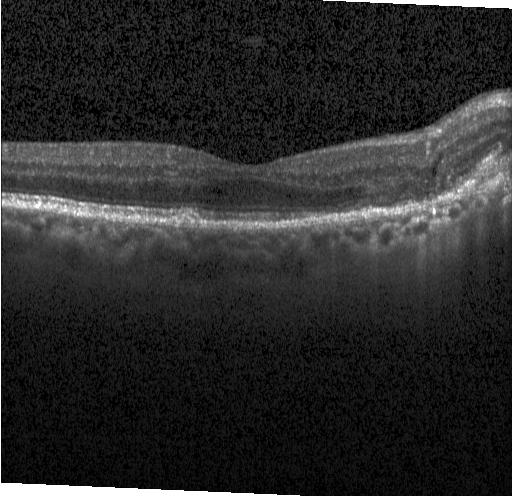 Heidelberg Spectralis. OCT B-scan
Diagnosis: a choroidal neovascular membrane.